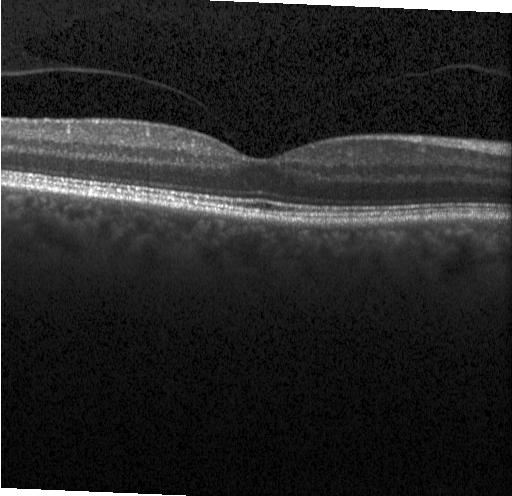
Retinal OCT B-scan
Impression: no evidence of choroidal neovascularization, diabetic macular edema, or drusen.